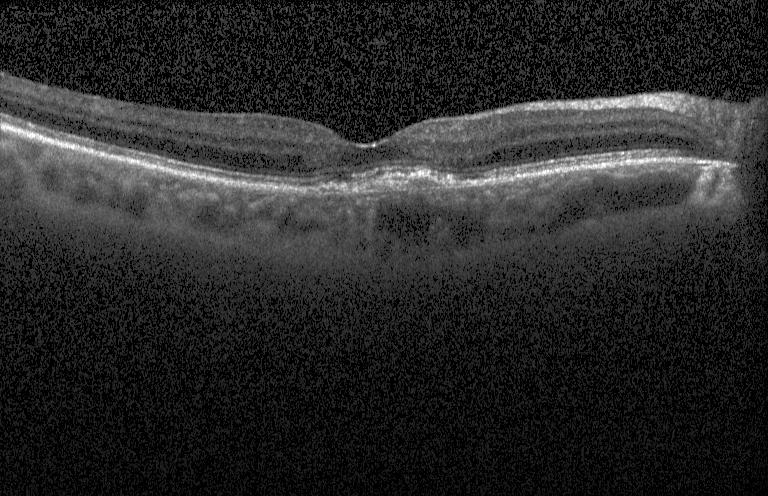

Diagnosis: choroidal neovascularization.